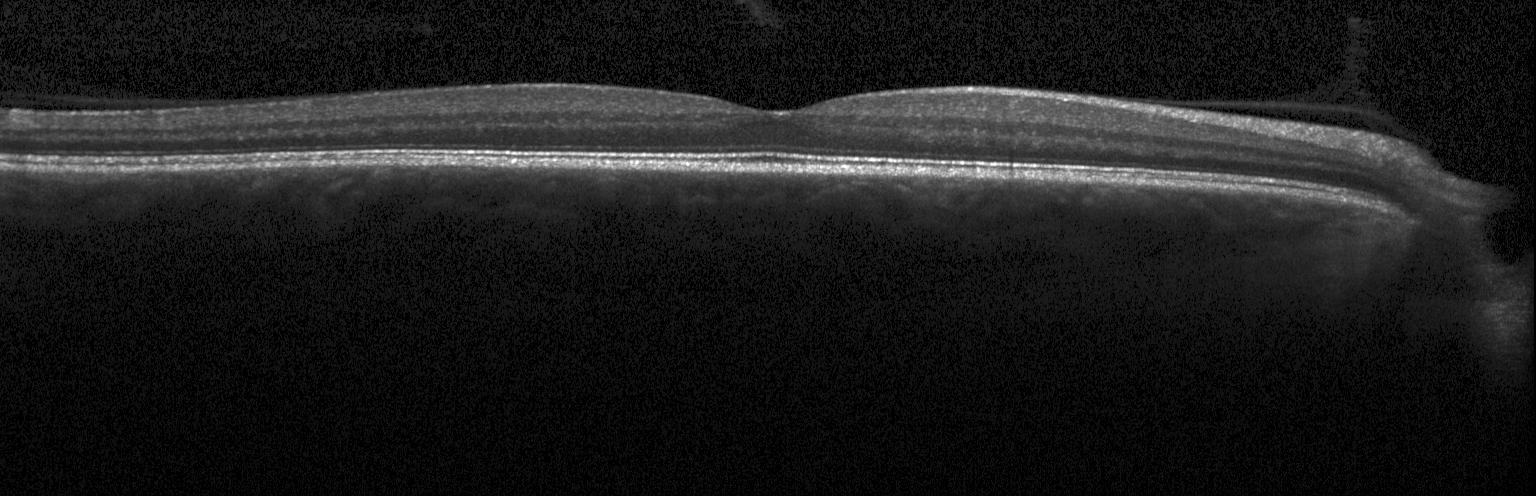 Optical coherence tomography scan · SD-OCT · fovea-centered. Finding: no CNV, no DME, and no drusen.